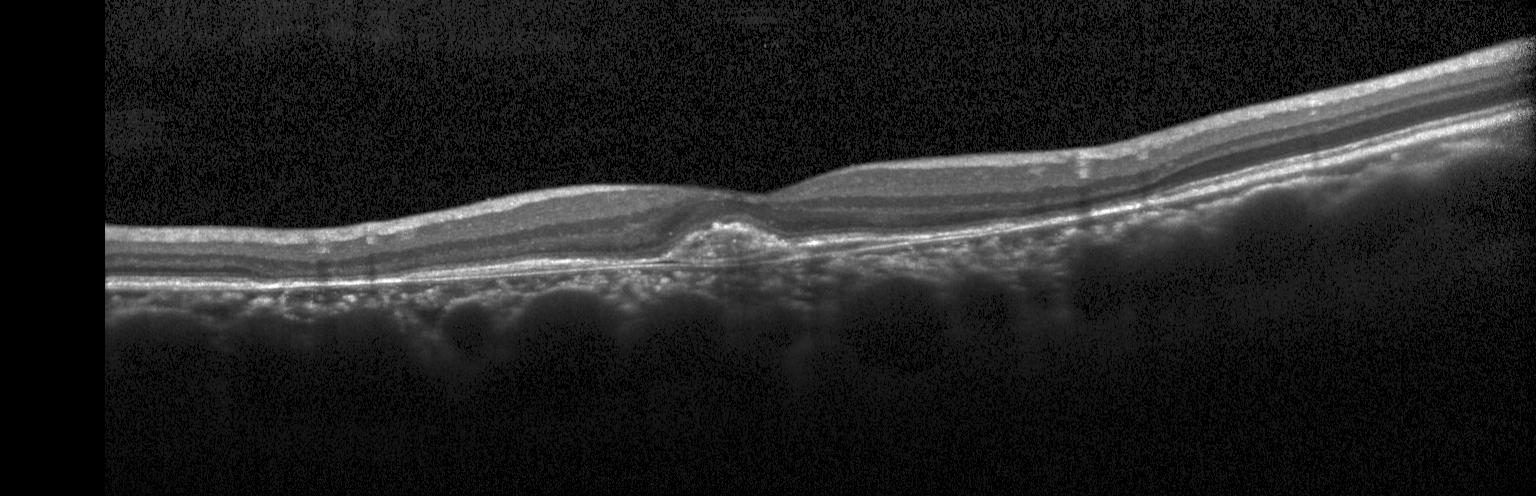 Acquired on a Heidelberg Spectralis; spectral-domain optical coherence tomography; optical coherence tomography B-scan; horizontal scan through the fovea. Macular OCT: a choroidal neovascular membrane.